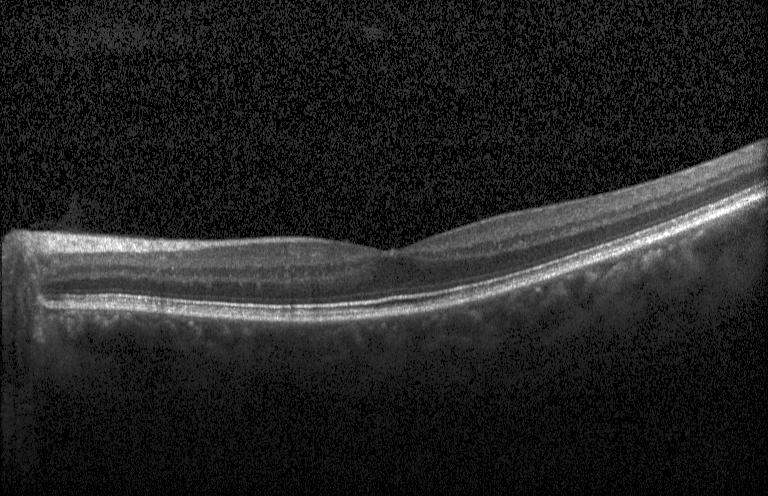
Macular OCT: no CNV, DME, or drusen.